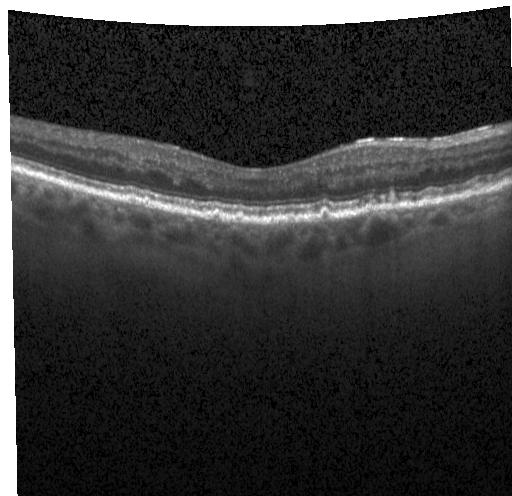
Dx: sub-RPE drusenoid deposits.